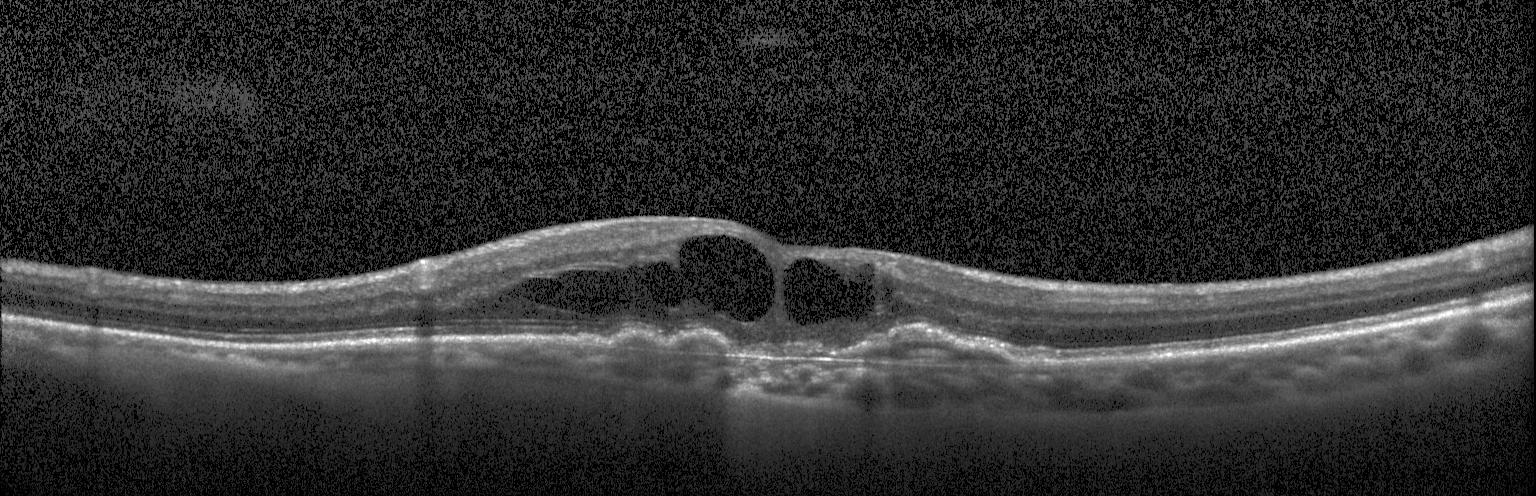 Retinal OCT B-scan. Heidelberg Spectralis.
Finding: a choroidal neovascular membrane.